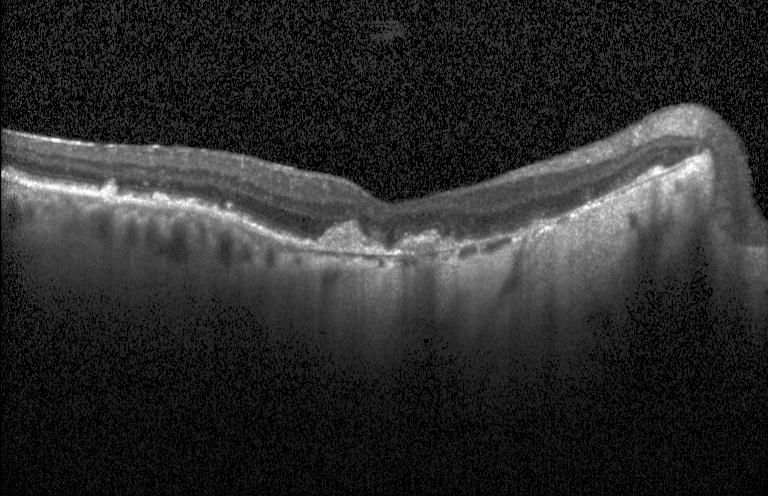

This B-scan demonstrates a choroidal neovascular membrane.